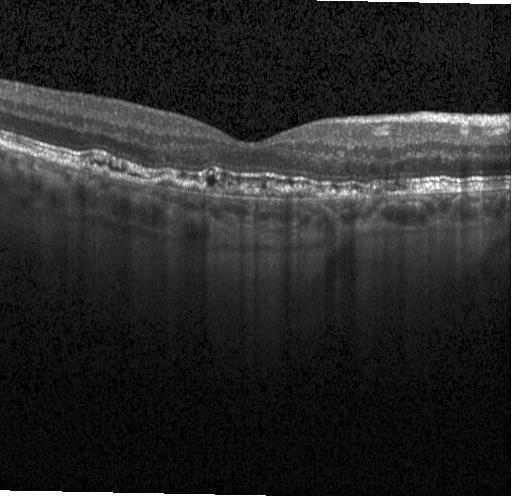
OCT B-scan — A choroidal neovascular membrane.